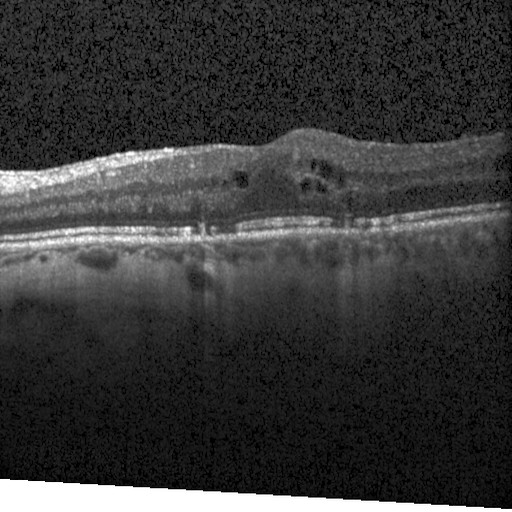

Instrument: Heidelberg Spectralis. OCT line scan. Fovea-centered. Diabetic macular edema.